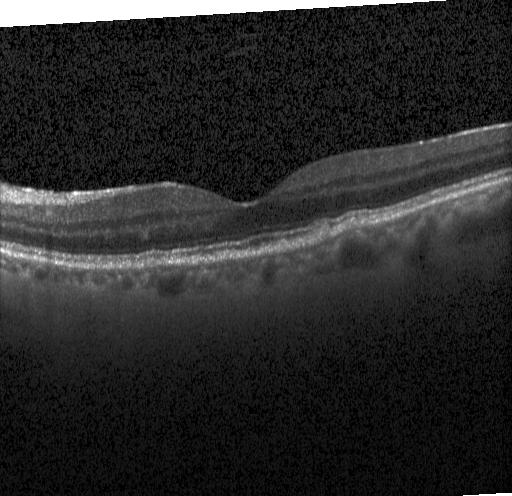
Dx: drusen.